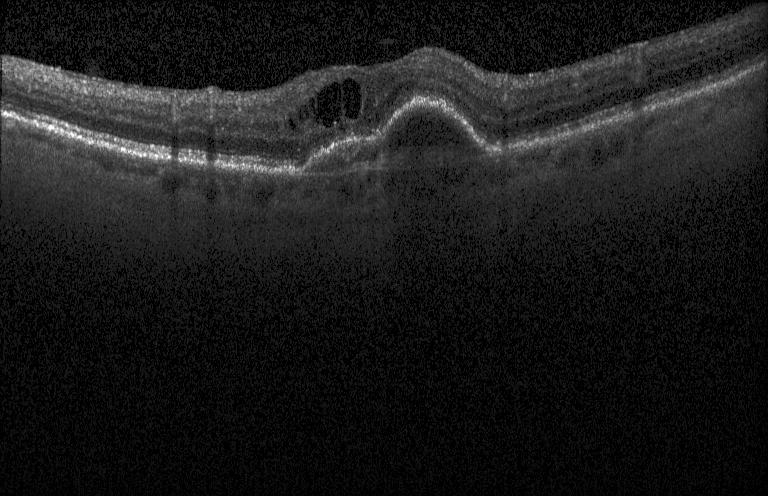
Retinal OCT B-scan.
Impression: a choroidal neovascular membrane.